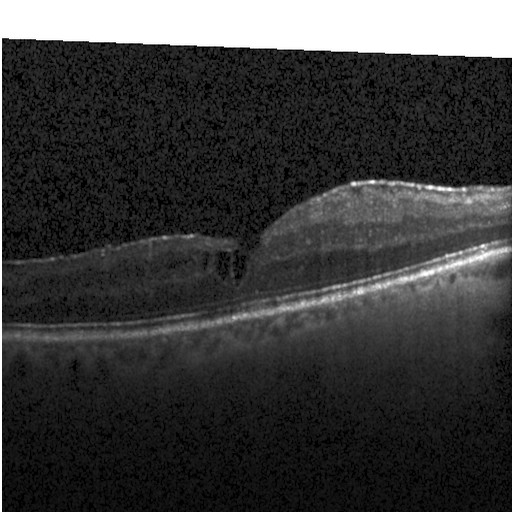
Finding: diabetic macular edema (DME).